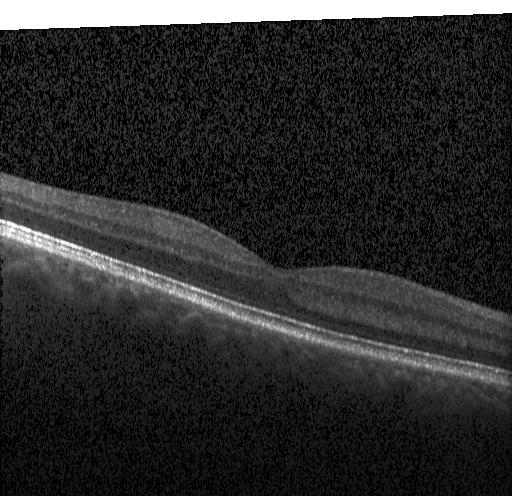
Instrument: Heidelberg Spectralis · optical coherence tomography B-scan · centered on the fovea.
The scan shows neither choroidal neovascularization, diabetic macular edema, nor drusen.